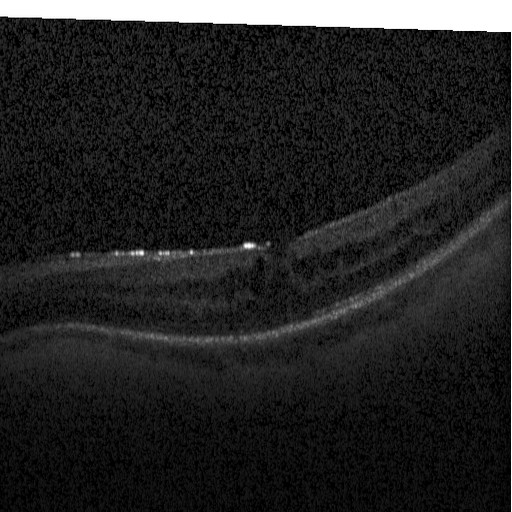
OCT scan showing DME.